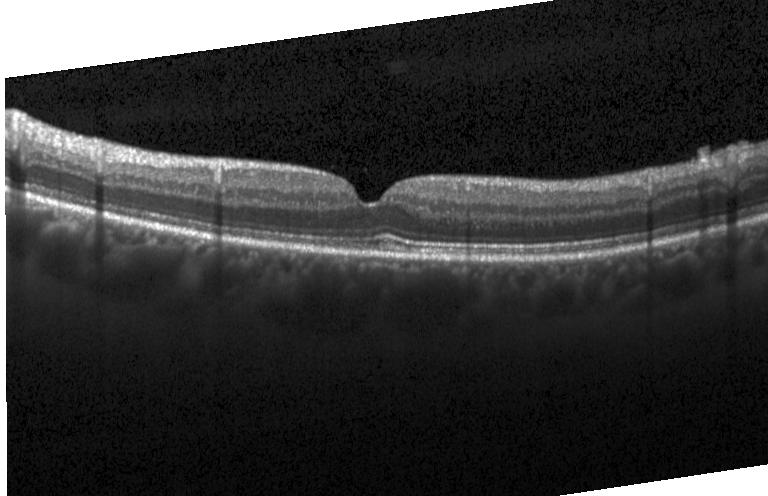

Optical coherence tomography B-scan.
Dx: no choroidal neovascularization, no diabetic macular edema, and no drusen.